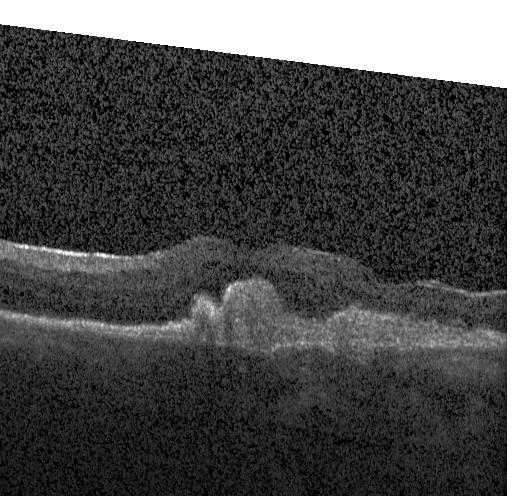
OCT finding: choroidal neovascularization.